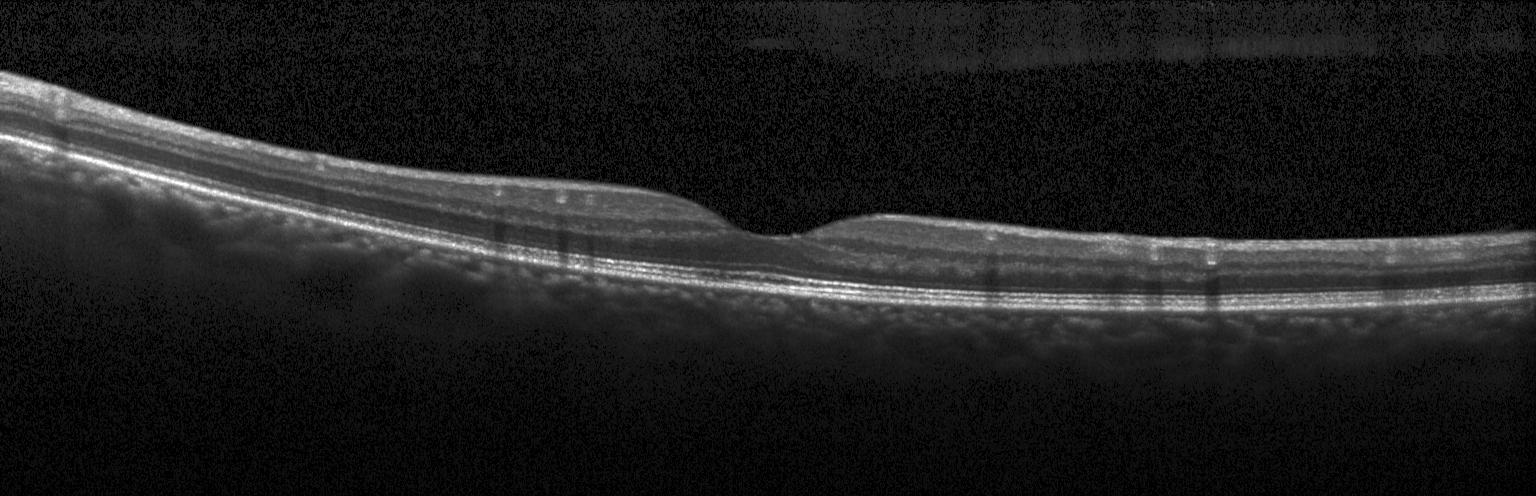

Retinal OCT cross-section; through the macula; instrument: Heidelberg Spectralis. The scan shows neither choroidal neovascularization, diabetic macular edema, nor drusen.